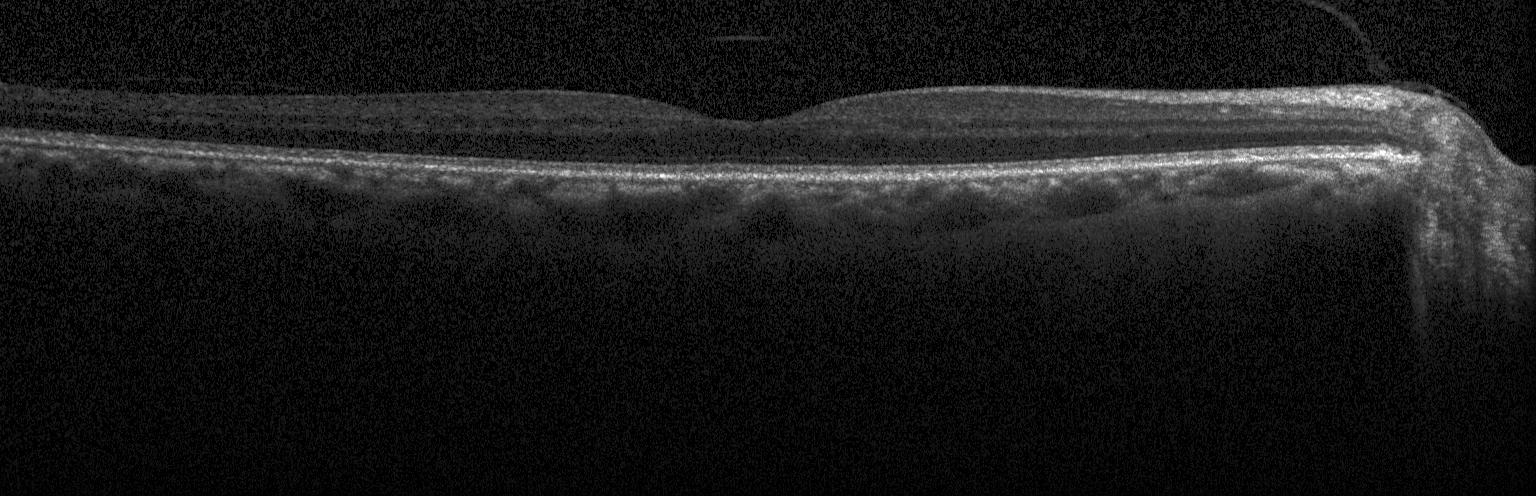 Diagnosis: no choroidal neovascularization, no diabetic macular edema, and no drusen.